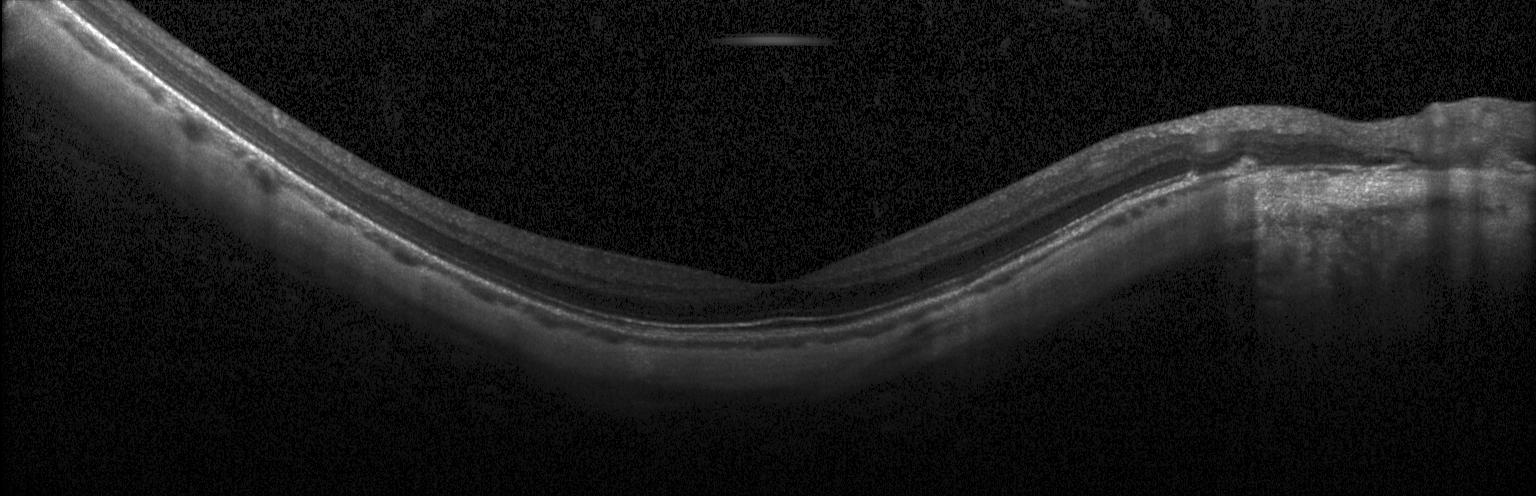

OCT scan showing no choroidal neovascularization, diabetic macular edema, or drusen.